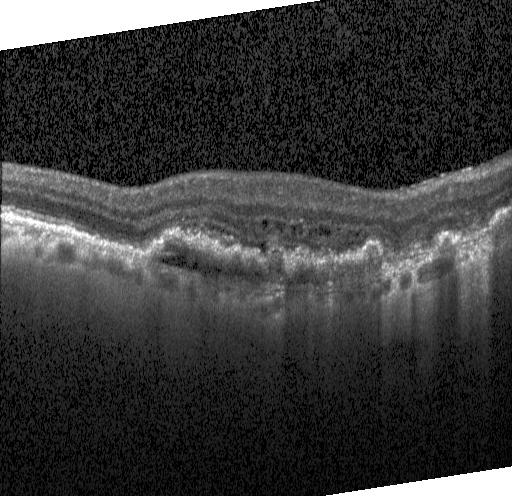

Optical coherence tomography scan. Macular scan. Heidelberg Spectralis OCT system.
Diagnosis: choroidal neovascularization (CNV).